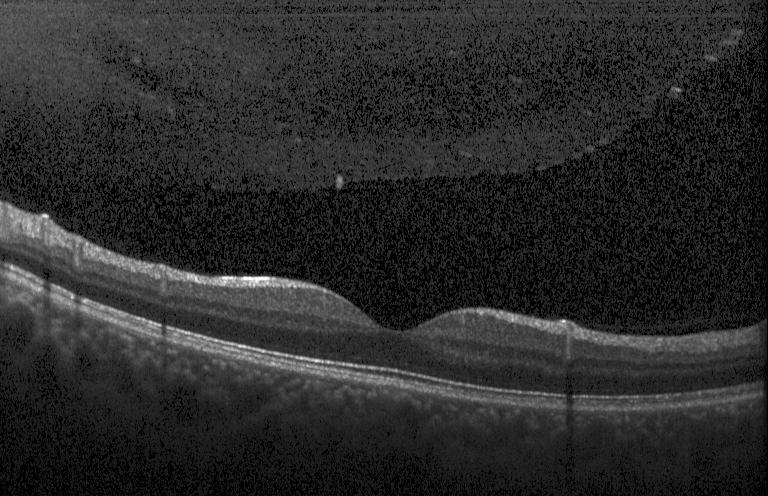
SD-OCT; Heidelberg Spectralis OCT system; optical coherence tomography B-scan. The scan shows neither choroidal neovascularization, diabetic macular edema, nor drusen.